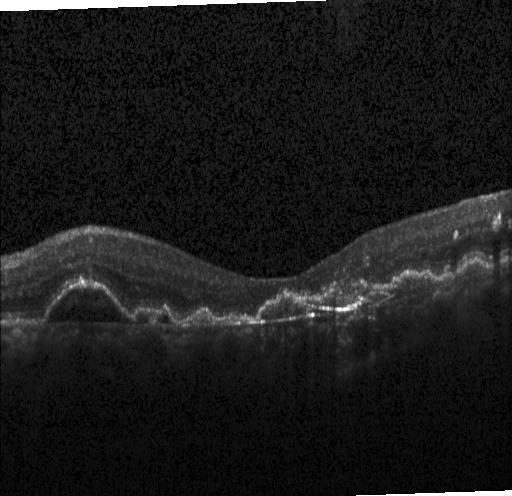 Spectral-domain OCT. Centered on the fovea. Optical coherence tomography scan. Heidelberg Spectralis OCT system.
This B-scan demonstrates a choroidal neovascular membrane.